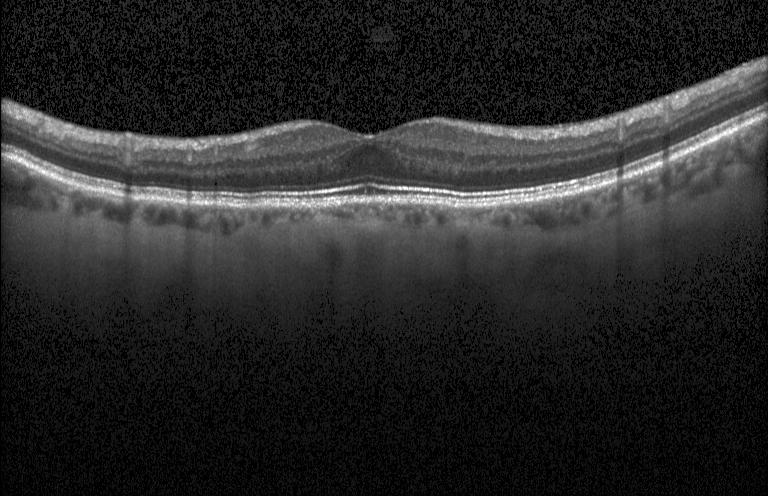 OCT B-scan; Heidelberg Spectralis OCT system; spectral-domain optical coherence tomography
This B-scan demonstrates no evidence of choroidal neovascularization, diabetic macular edema, or drusen.